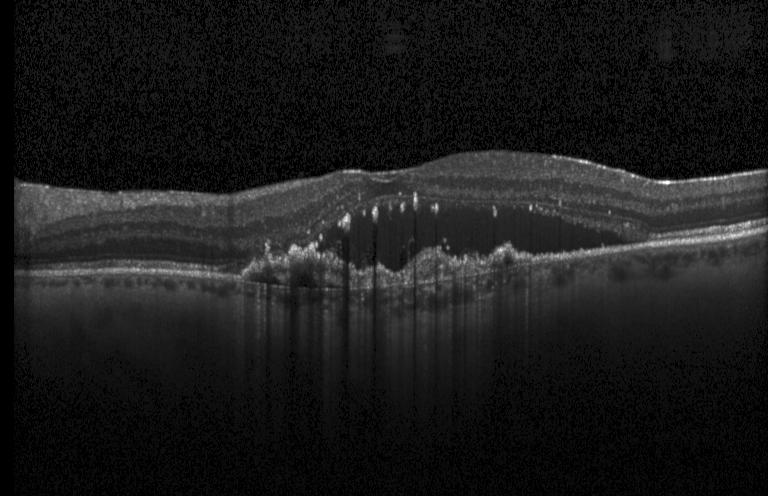

Impression: a choroidal neovascular membrane.